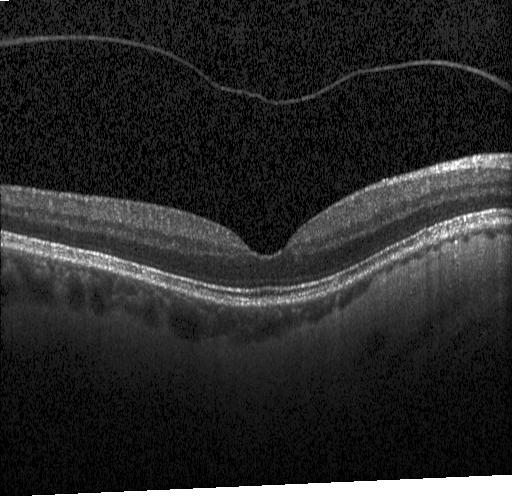

Diagnosis: no choroidal neovascularization, no diabetic macular edema, and no drusen.